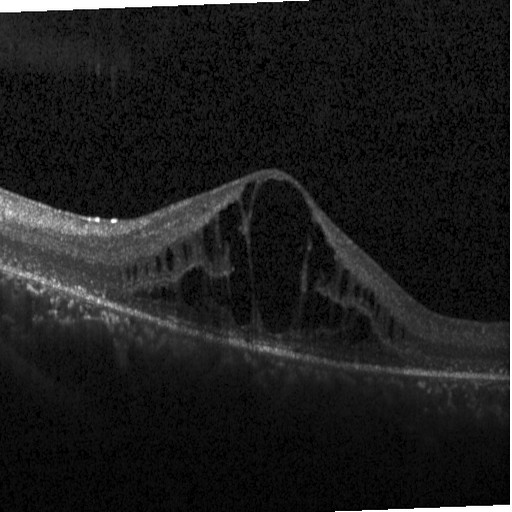

This B-scan demonstrates diabetic macular edema.